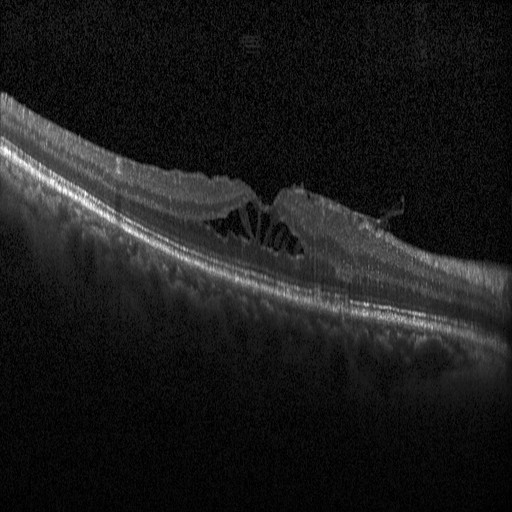 OCT line scan. Dx: DME.